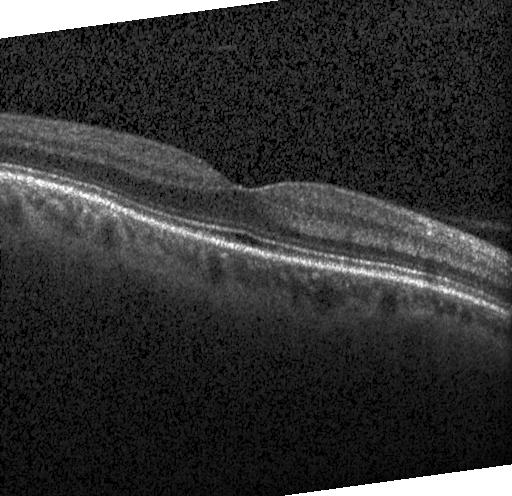

OCT B-scan showing no CNV, DME, or drusen.